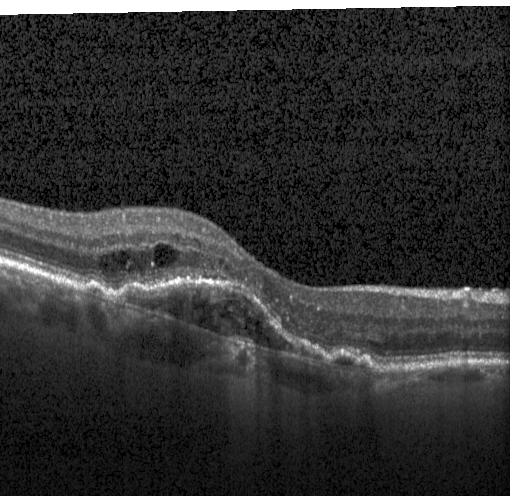 OCT line scan, spectral-domain OCT, horizontal scan through the fovea — Impression: choroidal neovascularization (CNV).